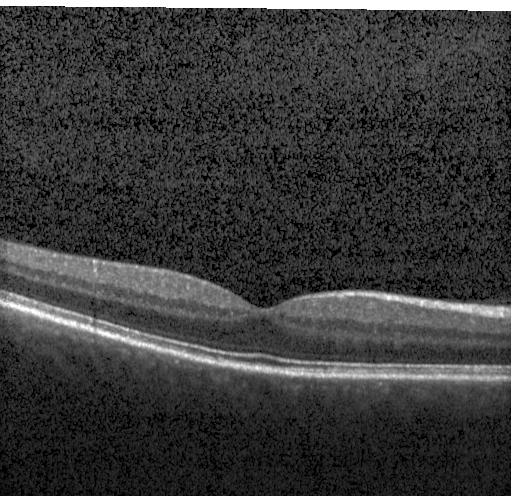
Diagnosis: no choroidal neovascularization, no diabetic macular edema, and no drusen.